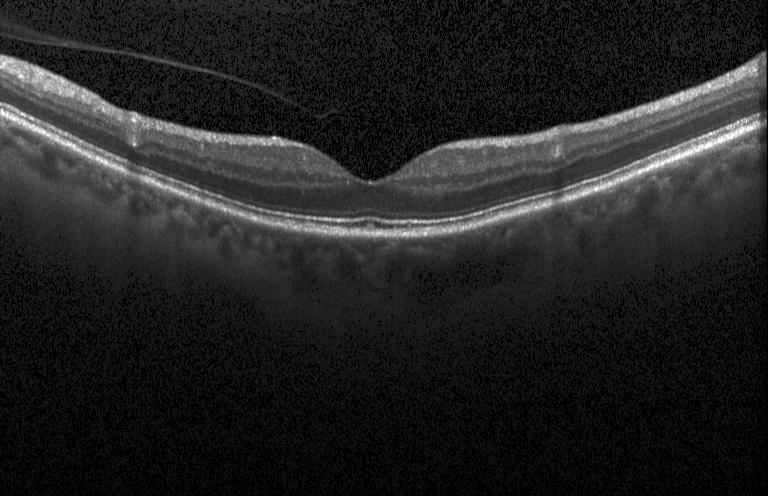
The scan shows neither CNV, DME, nor drusen.